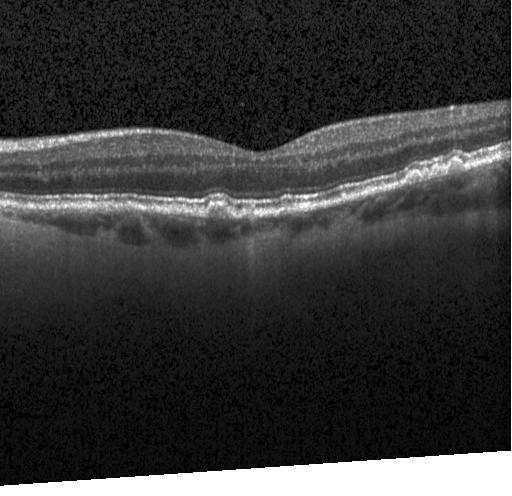
Finding: multiple drusen.